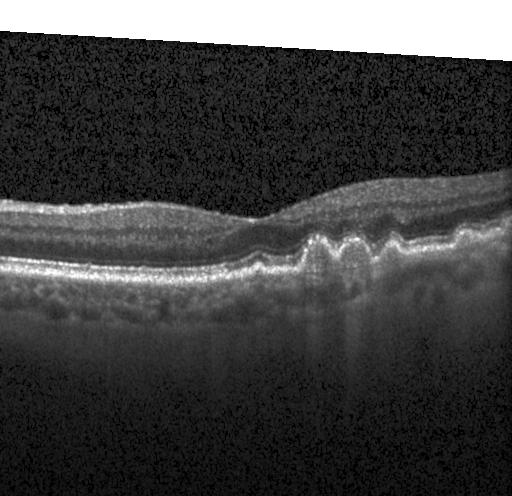

Heidelberg Spectralis, horizontal scan through the fovea, spectral-domain optical coherence tomography, optical coherence tomography scan — Finding: sub-RPE drusenoid deposits.